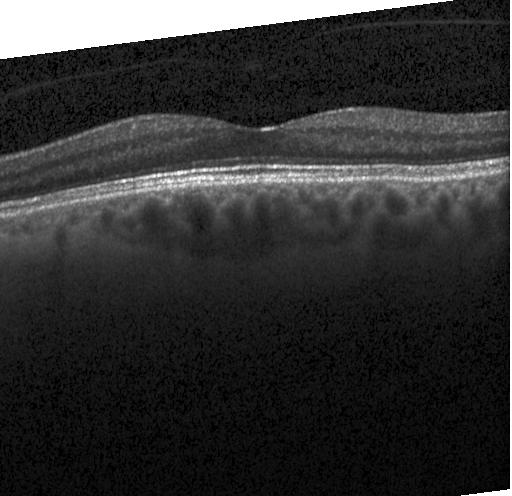 Retinal OCT cross-section showing no CNV, no DME, and no drusen.